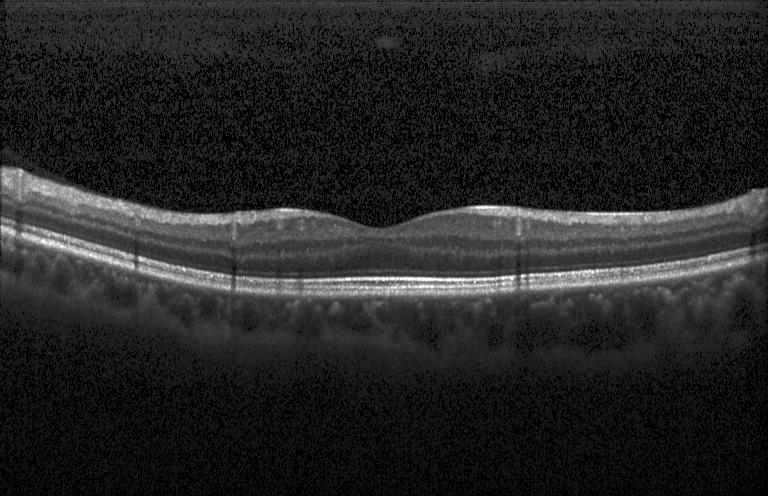 Diagnosis: no choroidal neovascularization, diabetic macular edema, or drusen.